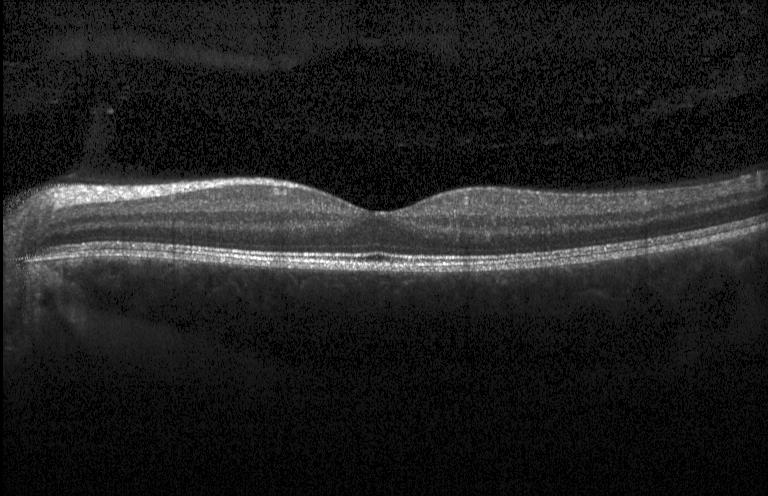
Optical coherence tomography B-scan. SD-OCT
Neither CNV, DME, nor drusen.